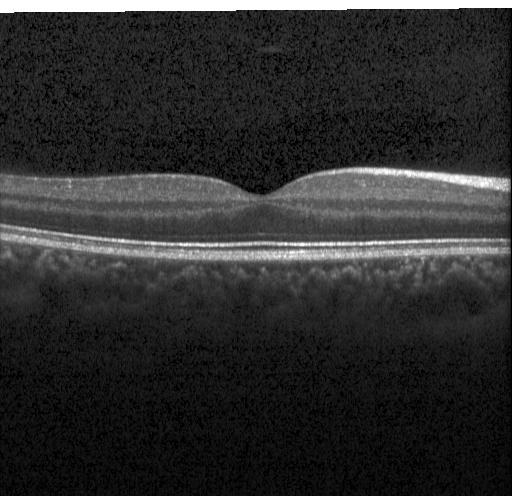 No choroidal neovascularization, diabetic macular edema, or drusen.